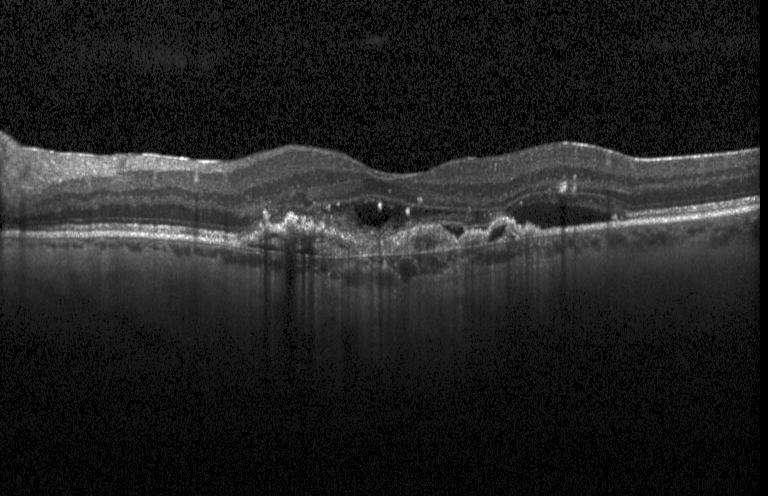 OCT line scan. Heidelberg Spectralis. Impression: a choroidal neovascular membrane.